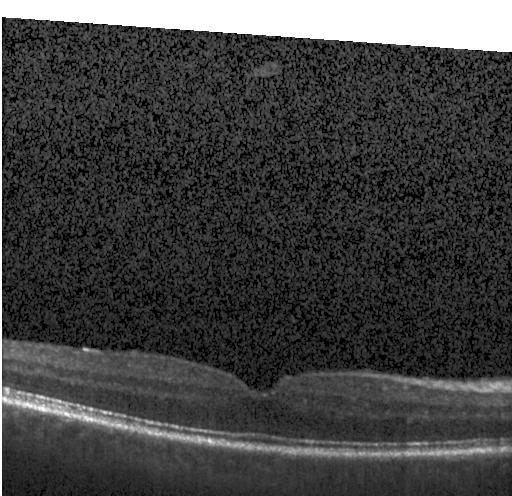
OCT finding: neither choroidal neovascularization, diabetic macular edema, nor drusen.